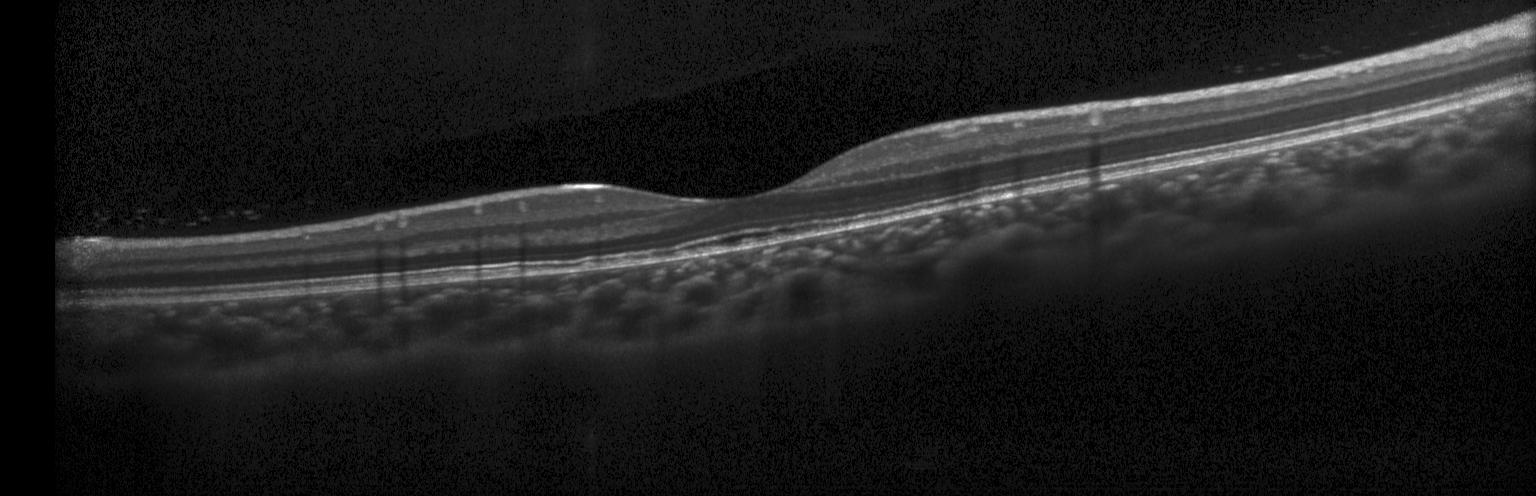 OCT line scan.
Finding: neither choroidal neovascularization, diabetic macular edema, nor drusen.